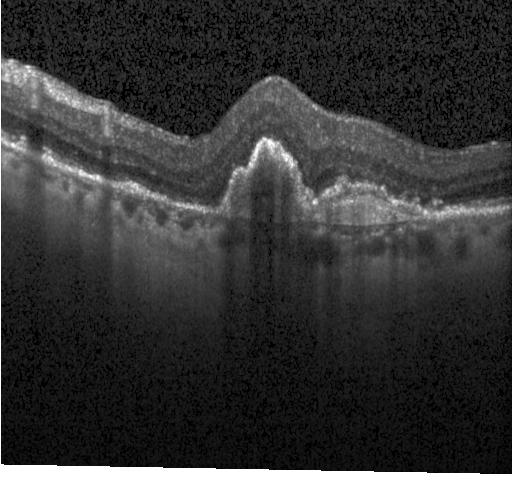
Assessment: choroidal neovascularization.